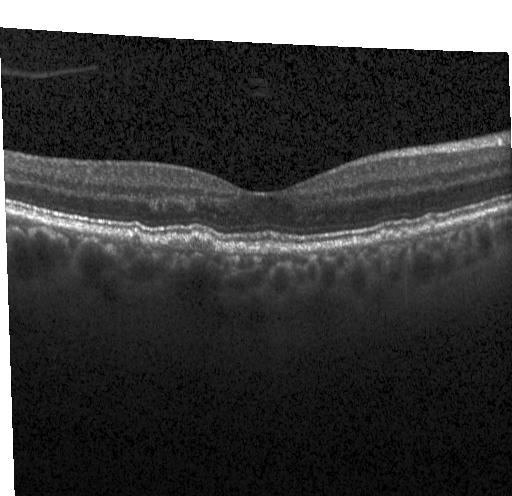 Heidelberg Spectralis · spectral-domain optical coherence tomography · optical coherence tomography B-scan.
Diagnosis: multiple drusen.